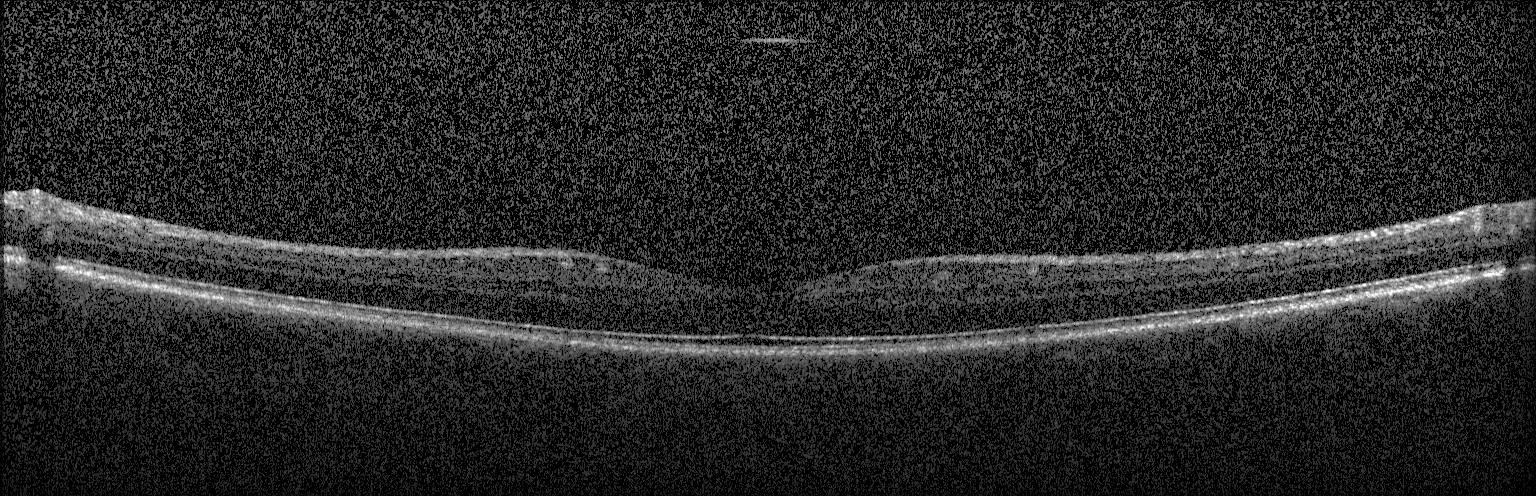 OCT B-scan; centered on the fovea — No choroidal neovascularization, no diabetic macular edema, and no drusen.